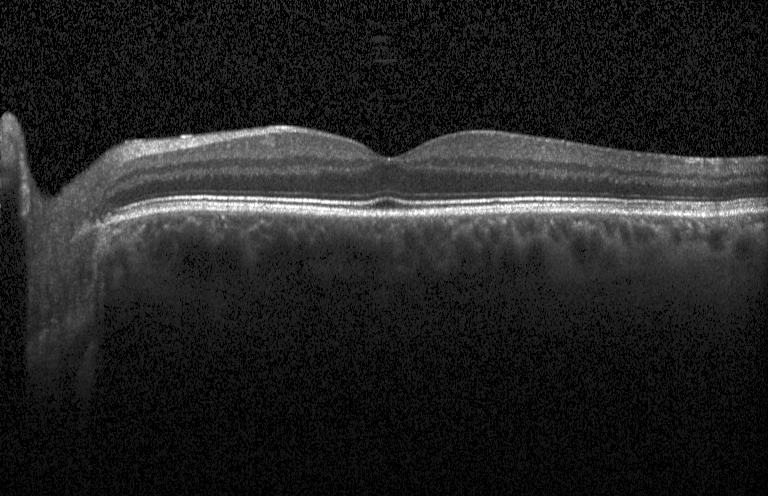
Optical coherence tomography B-scan. Instrument: Heidelberg Spectralis. Macular scan. Spectral-domain optical coherence tomography.
Neither CNV, DME, nor drusen.